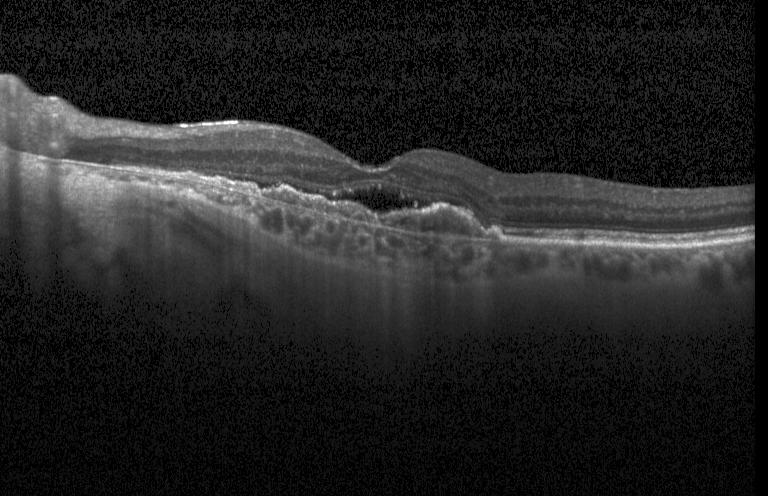

Dx: a choroidal neovascular membrane.